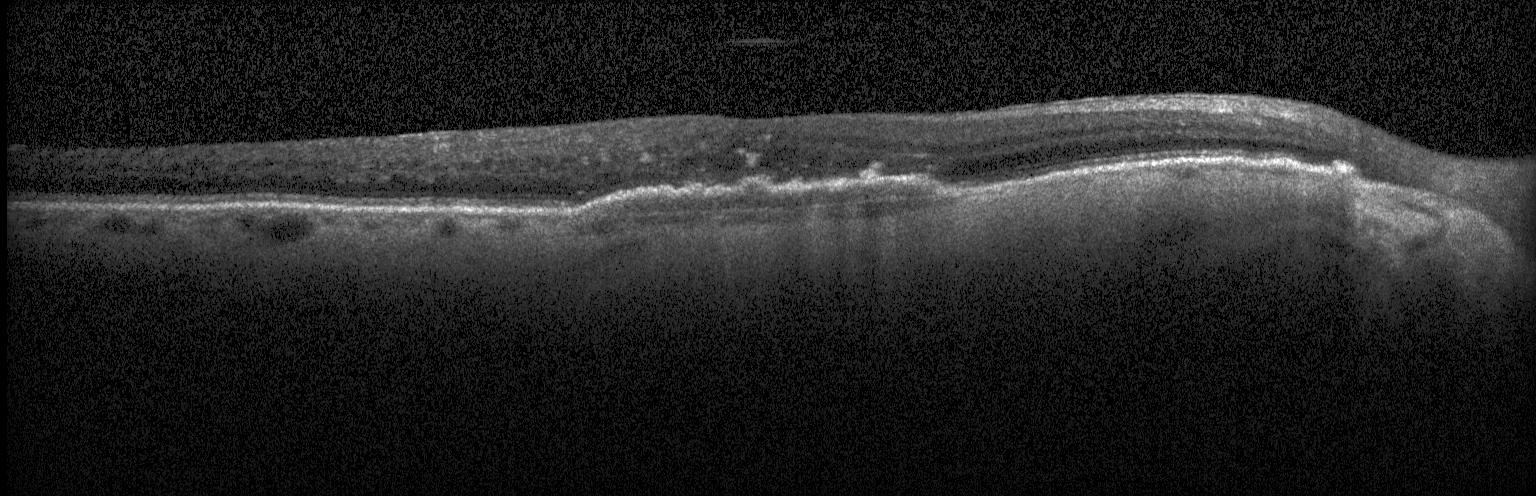 Heidelberg Spectralis OCT system · retinal OCT cross-section
Finding: a choroidal neovascular membrane.